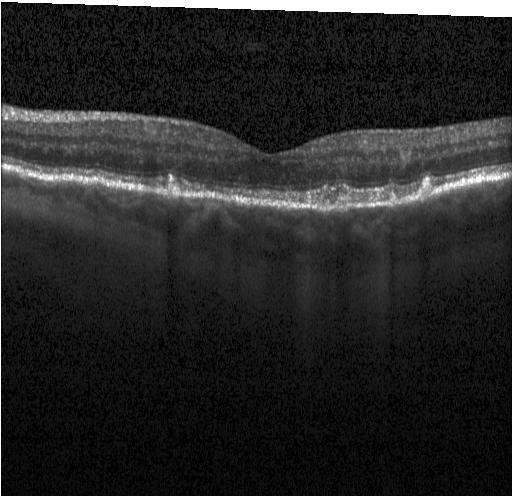

Diagnosis: multiple drusen.